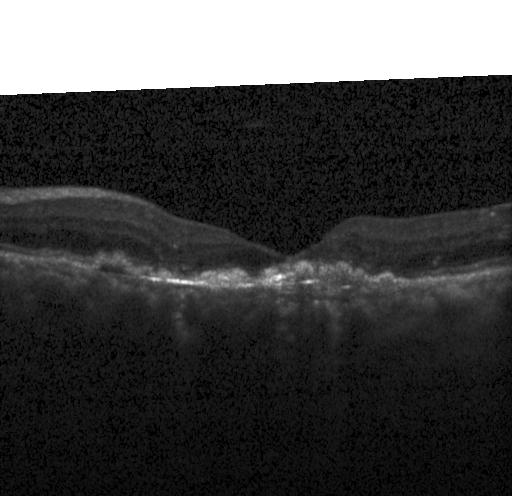

Macular OCT: CNV.